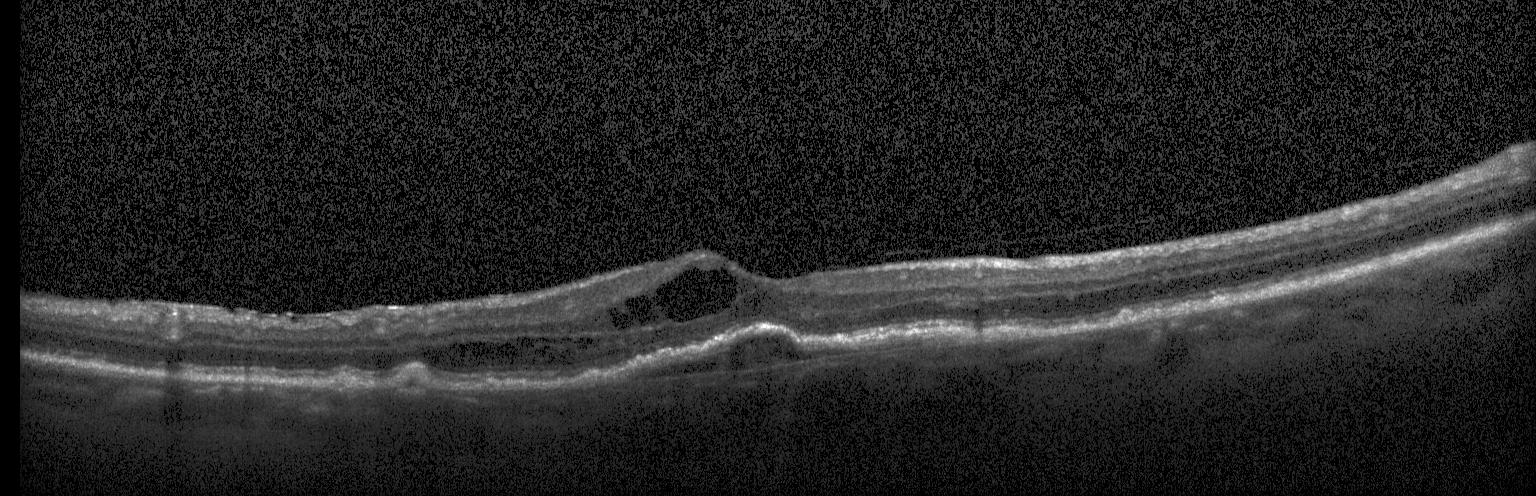 Finding: choroidal neovascularization (CNV).